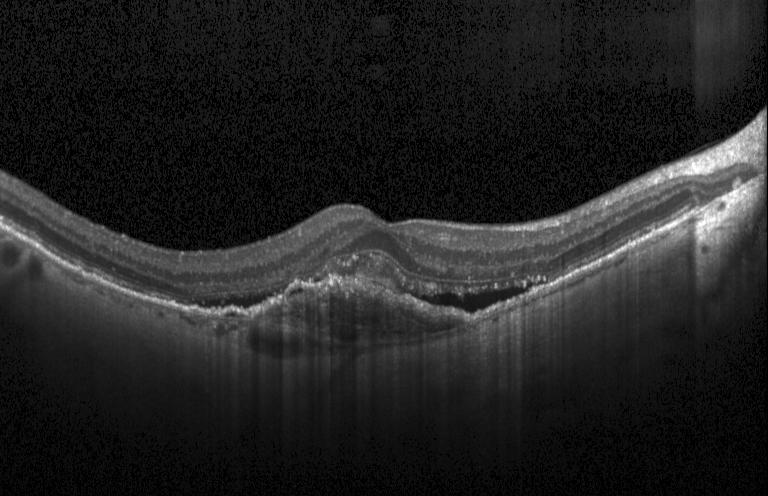
Spectral-domain OCT B-scan: a choroidal neovascular membrane.